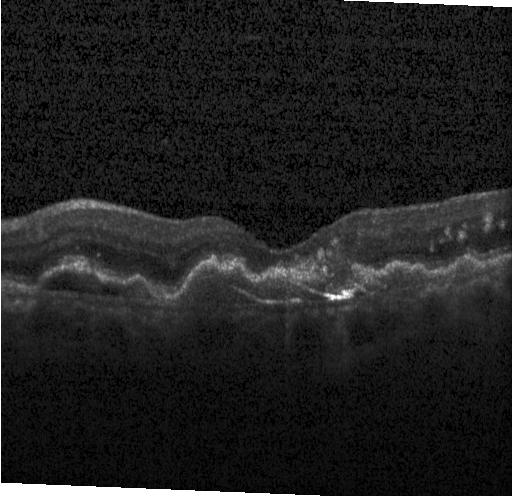 Optical coherence tomography B-scan. Finding: choroidal neovascularization (CNV).